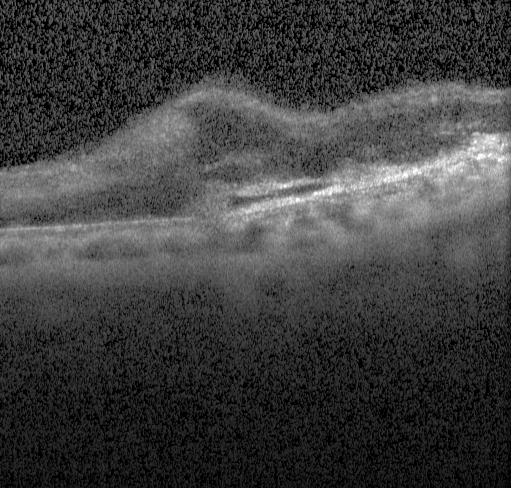

OCT line scan.
Diagnosis: a choroidal neovascular membrane.